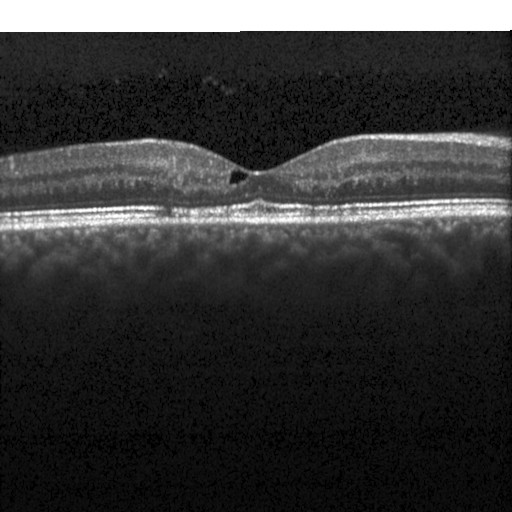

Retinal OCT B-scan · instrument: Heidelberg Spectralis · SD-OCT — Diagnosis: diabetic macular edema.